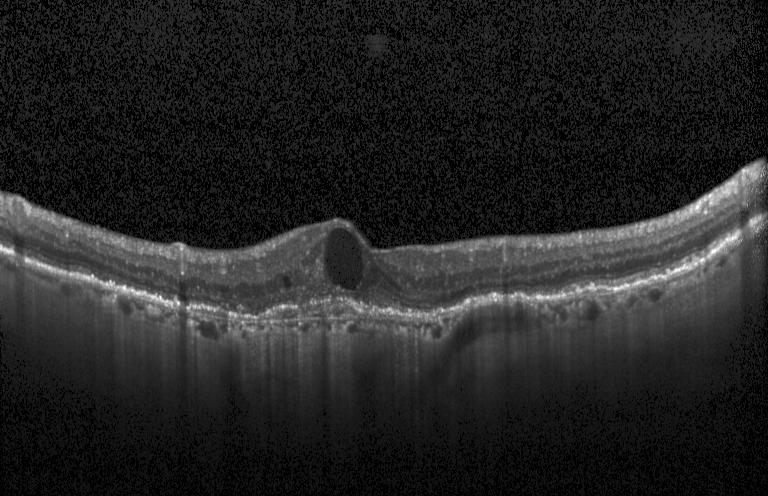

Optical coherence tomography B-scan
Assessment: choroidal neovascularization (CNV).